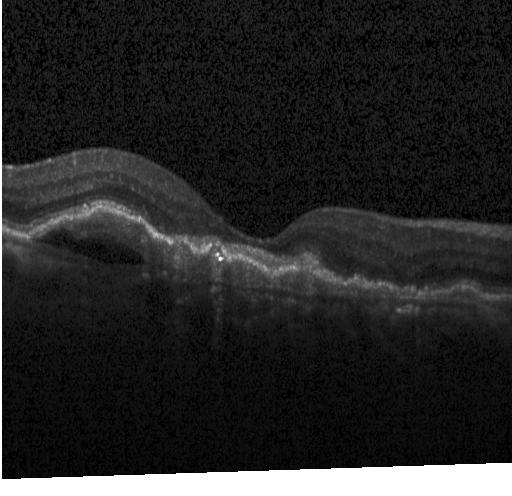
Retinal OCT cross-section showing a choroidal neovascular membrane.